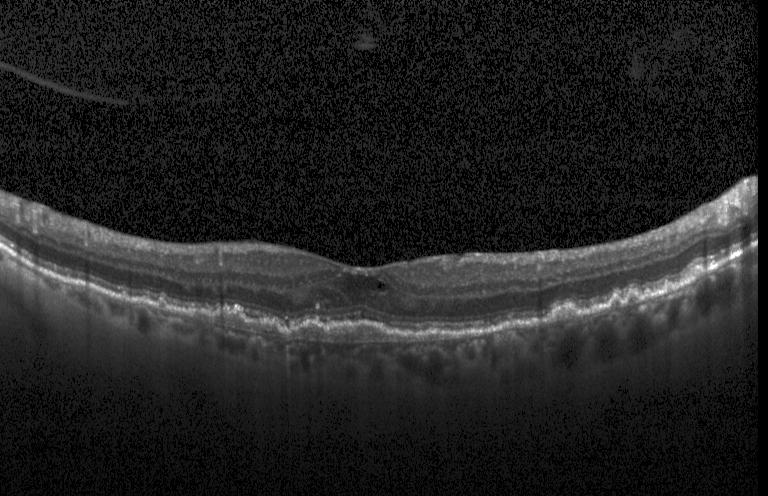 OCT B-scan
Impression: CNV.